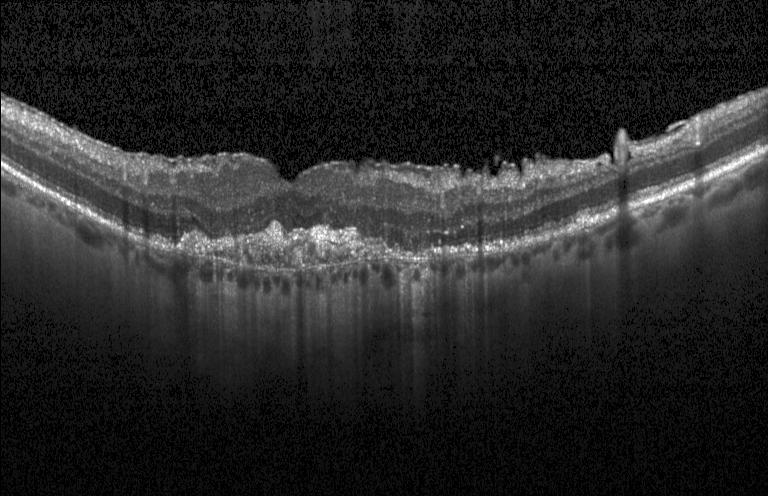 Optical coherence tomography scan. Dx: a choroidal neovascular membrane.